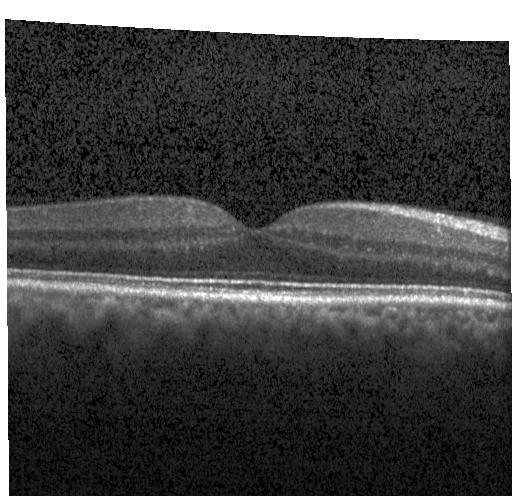

Retinal OCT cross-section — Finding: neither CNV, DME, nor drusen.